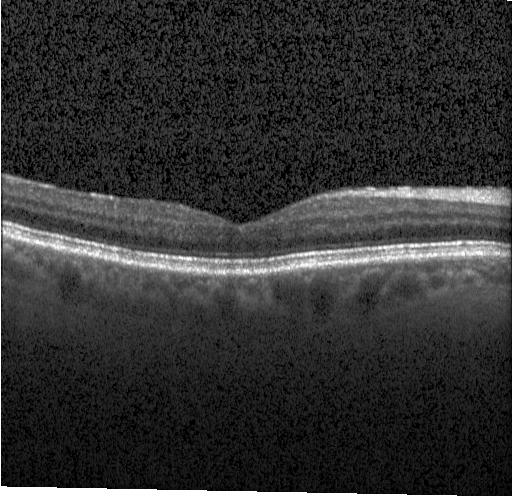

Finding: no evidence of choroidal neovascularization, diabetic macular edema, or drusen.